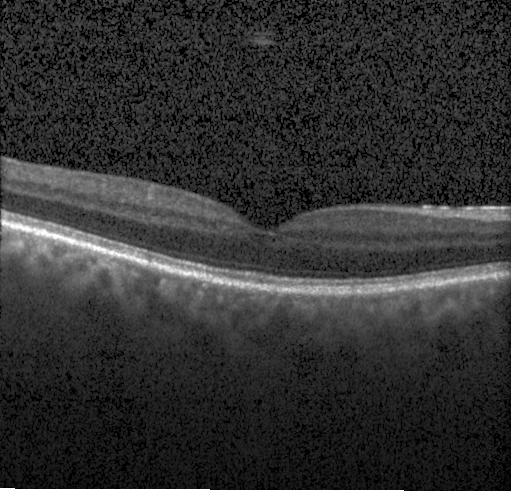
Retinal OCT cross-section. Spectral-domain OCT. Horizontal scan through the fovea. Heidelberg Spectralis. Impression: no choroidal neovascularization, no diabetic macular edema, and no drusen.